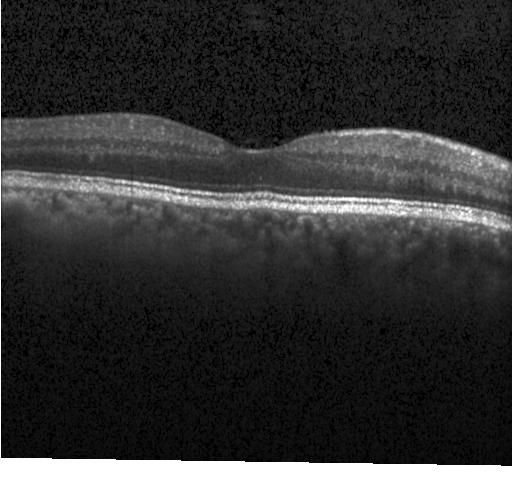 Heidelberg Spectralis OCT system; centered on the fovea; spectral-domain OCT; retinal OCT B-scan — Impression: no evidence of choroidal neovascularization, diabetic macular edema, or drusen.